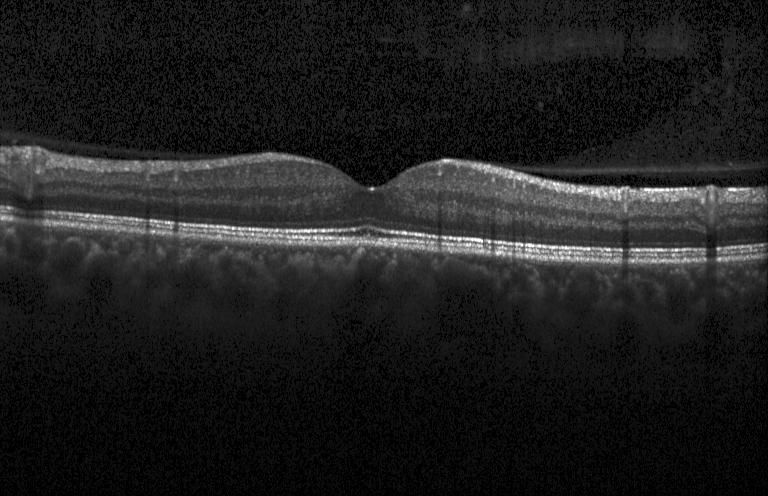

Instrument: Heidelberg Spectralis. OCT B-scan. Centered on the fovea. SD-OCT. Assessment: neither choroidal neovascularization, diabetic macular edema, nor drusen.